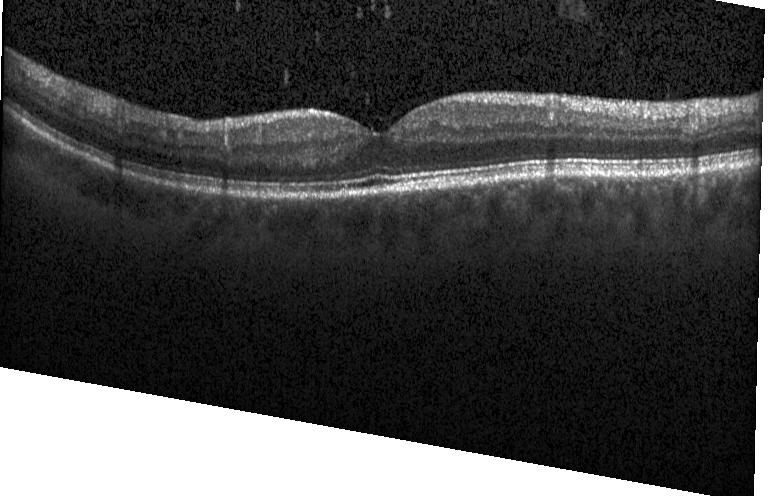
Finding: no choroidal neovascularization, diabetic macular edema, or drusen.